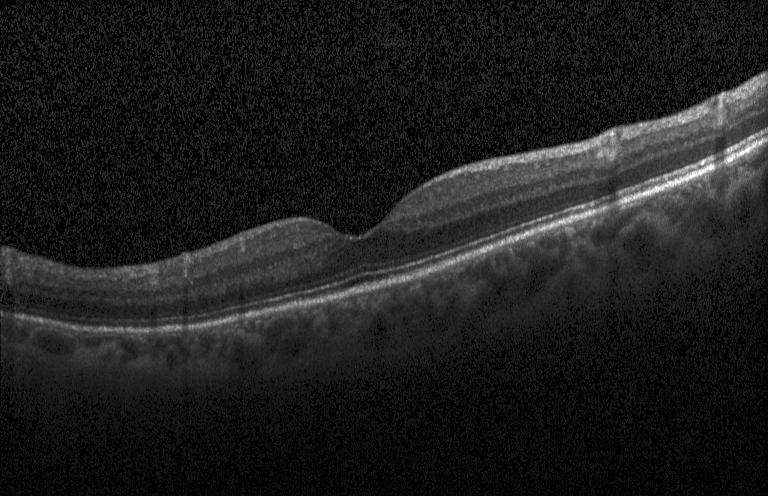 Spectral-domain optical coherence tomography. Heidelberg Spectralis OCT system. OCT B-scan. Macular scan.
Diagnosis: neither choroidal neovascularization, diabetic macular edema, nor drusen.